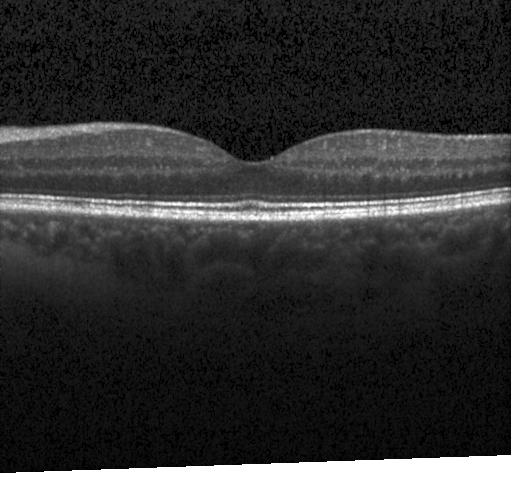
SD-OCT; OCT line scan; instrument: Heidelberg Spectralis — No evidence of choroidal neovascularization, diabetic macular edema, or drusen.